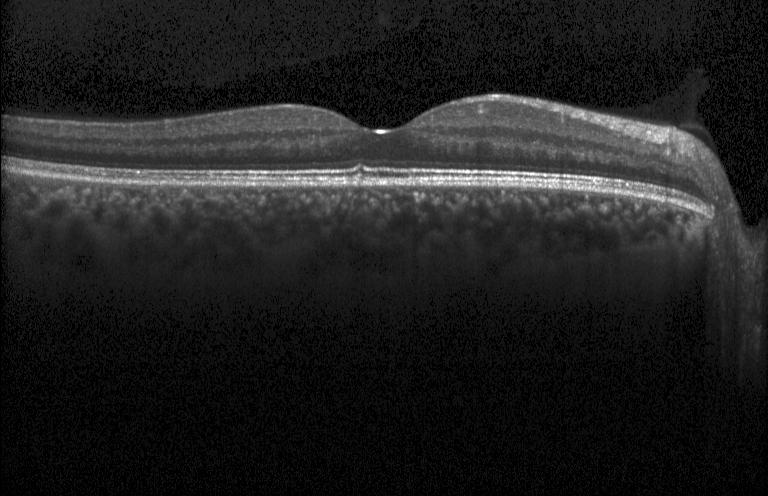
SD-OCT · OCT line scan · fovea-centered — OCT finding: drusen.